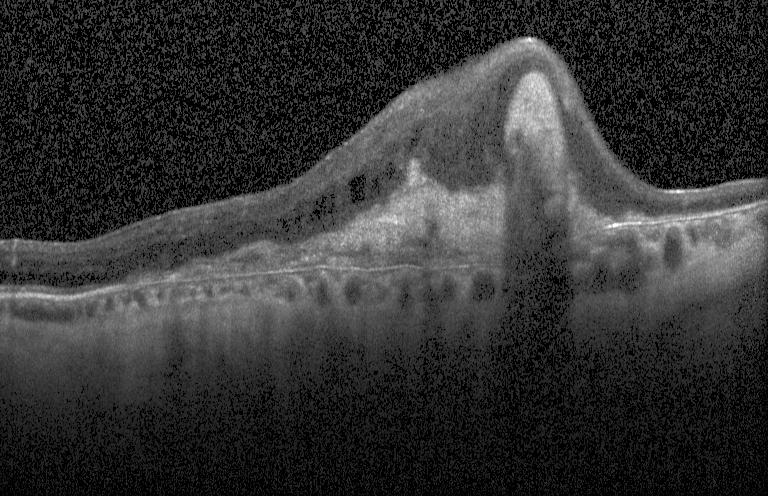
OCT B-scan showing CNV.